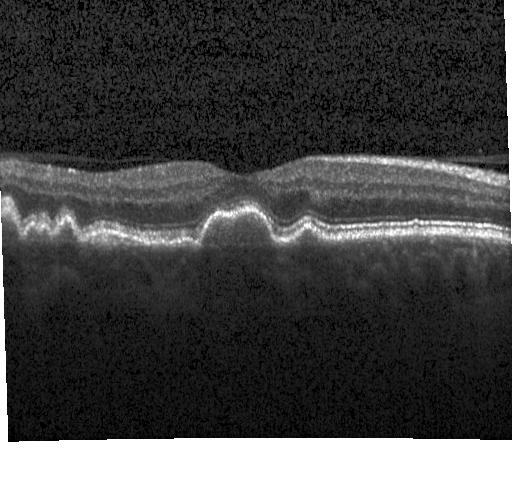

Optical coherence tomography B-scan
Macular OCT: drusen.